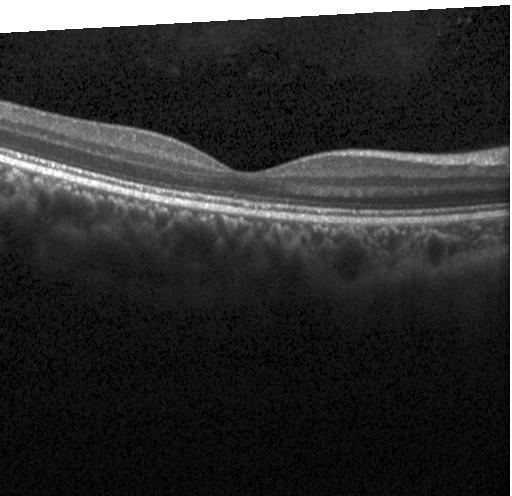
Spectral-domain OCT; optical coherence tomography scan; acquired on a Heidelberg Spectralis; horizontal scan through the fovea — Impression: no CNV, DME, or drusen.